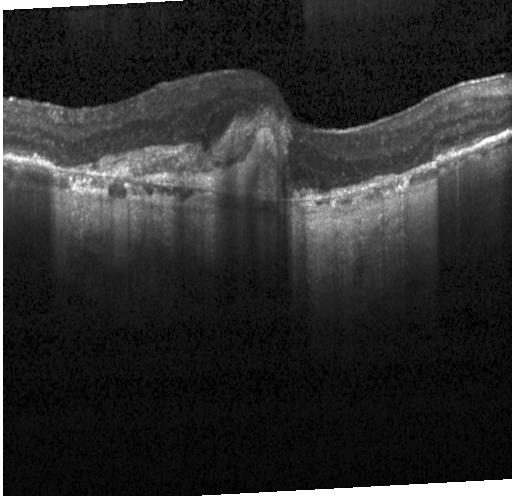

Retinal OCT cross-section. Macular scan.
Diagnosis: choroidal neovascularization (CNV).